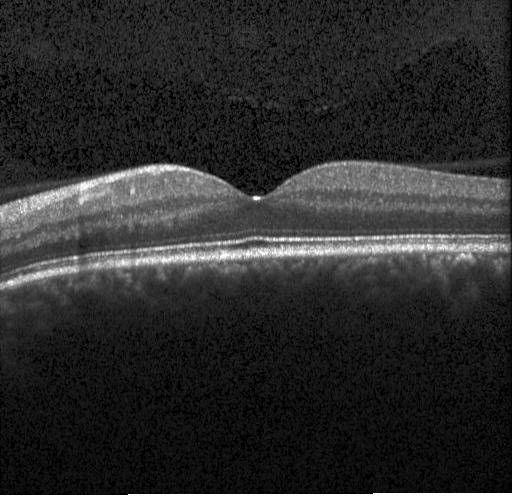
Fovea-centered; Heidelberg Spectralis; spectral-domain OCT; retinal OCT B-scan — Impression: no CNV, no DME, and no drusen.